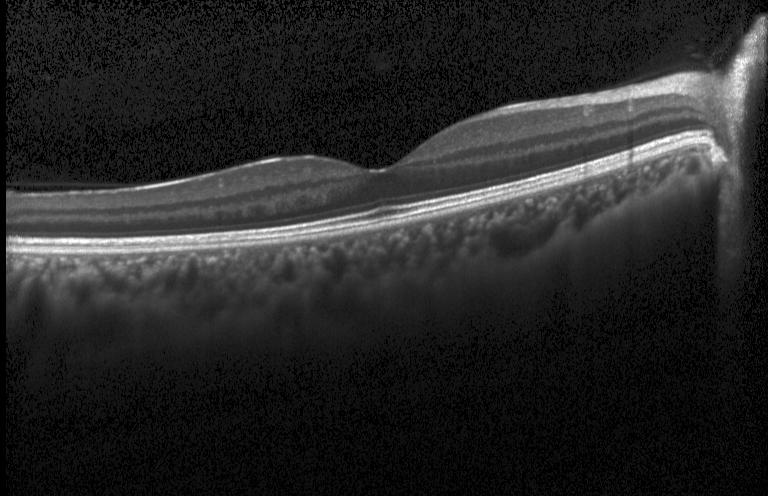

Diagnosis: no CNV, DME, or drusen.